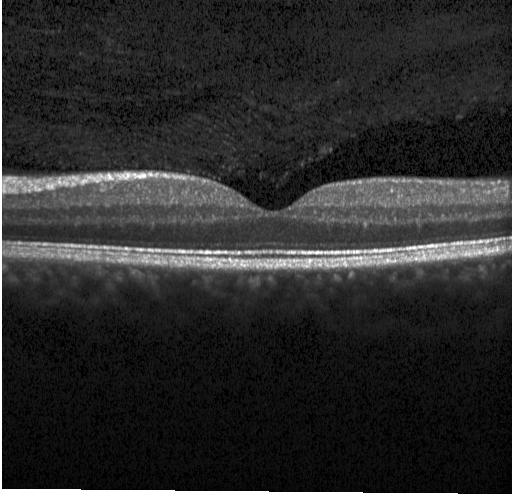

Heidelberg Spectralis OCT system; OCT B-scan; centered on the fovea. Finding: no choroidal neovascularization, diabetic macular edema, or drusen.